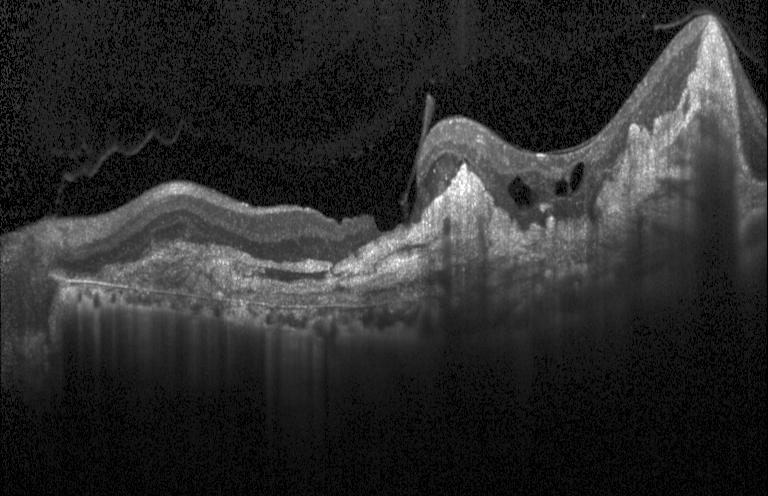

Retinal OCT B-scan. Dx: a choroidal neovascular membrane.